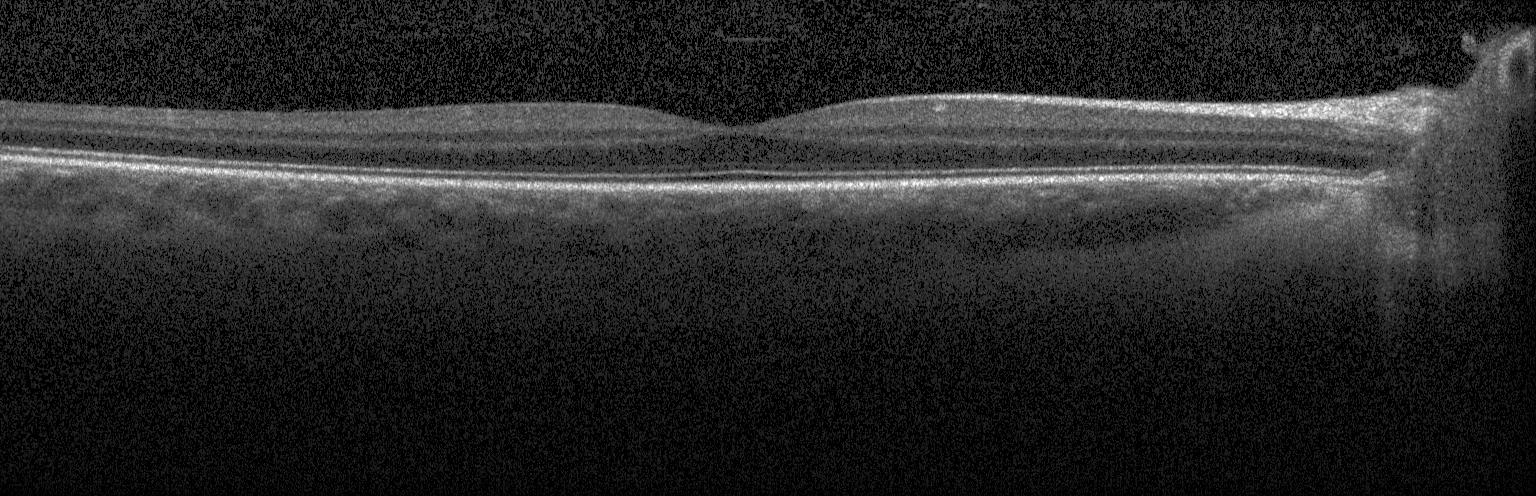
Optical coherence tomography B-scan
OCT finding: no evidence of choroidal neovascularization, diabetic macular edema, or drusen.